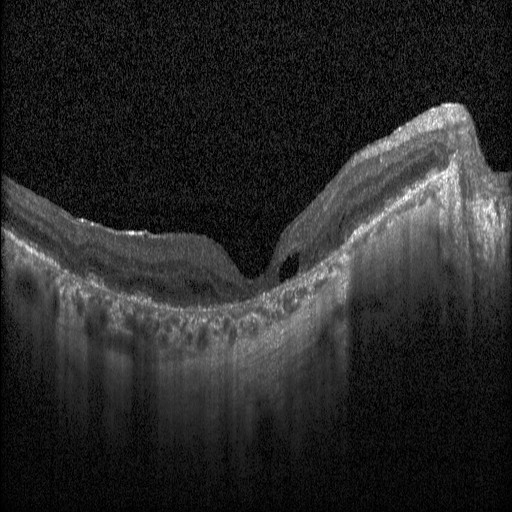

OCT B-scan · instrument: Heidelberg Spectralis. Impression: diabetic macular edema (DME).